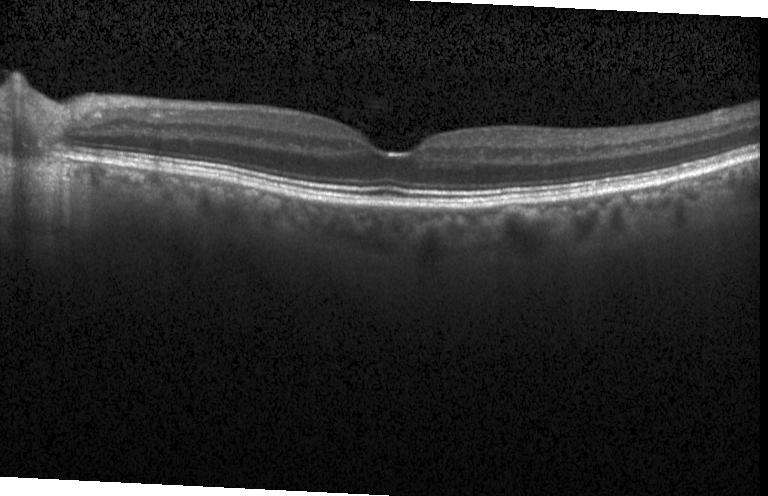

Retinal OCT B-scan · SD-OCT · instrument: Heidelberg Spectralis · through the macula
Dx: neither CNV, DME, nor drusen.